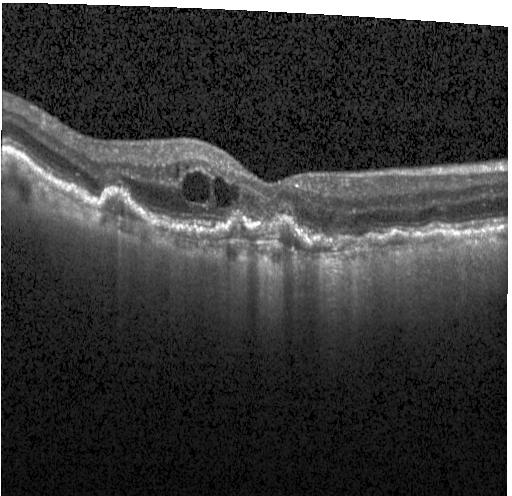

Impression: a choroidal neovascular membrane.